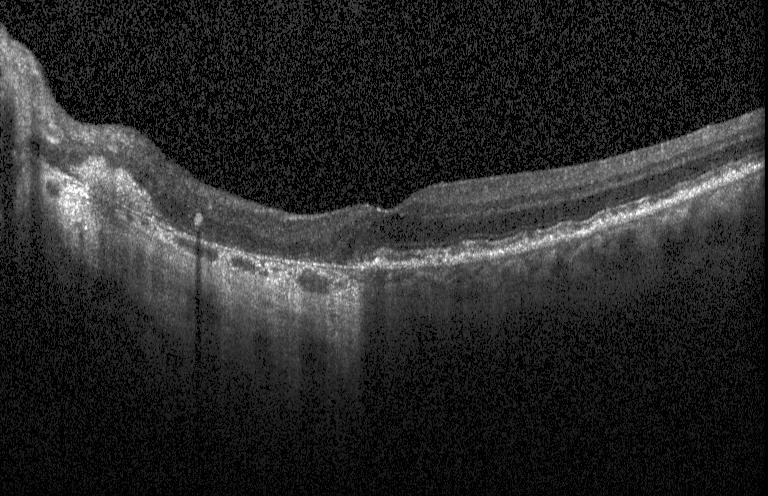

SD-OCT. Heidelberg Spectralis OCT system. OCT B-scan. Impression: a choroidal neovascular membrane.